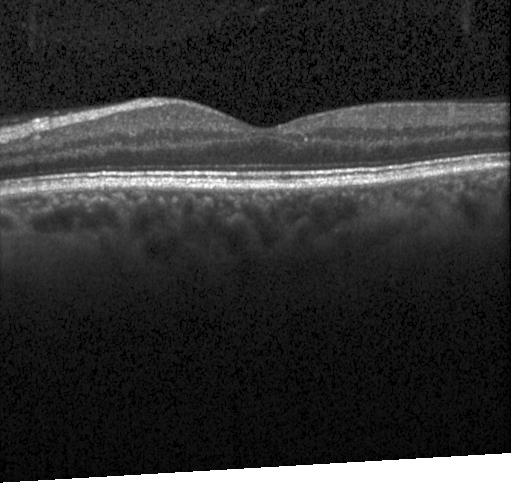
Macular scan · Heidelberg Spectralis OCT system · SD-OCT · optical coherence tomography B-scan.
OCT finding: no choroidal neovascularization, diabetic macular edema, or drusen.